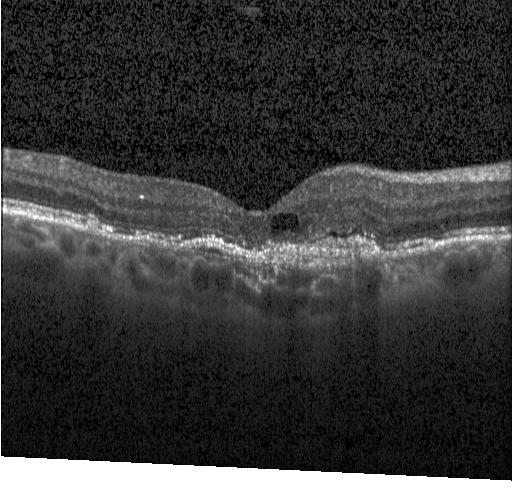
OCT B-scan showing a choroidal neovascular membrane.